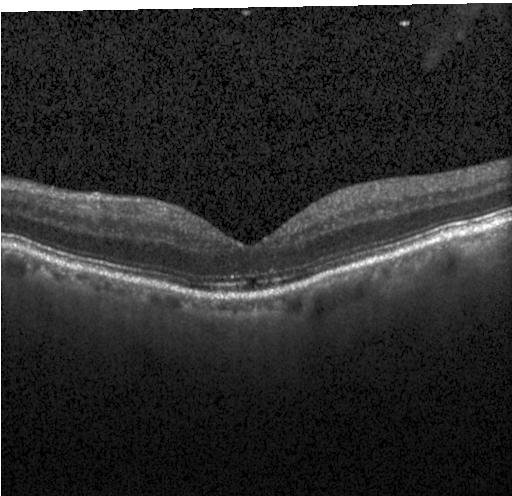 OCT line scan · Heidelberg Spectralis OCT system · macular scan · spectral-domain optical coherence tomography
Diagnosis: no choroidal neovascularization, diabetic macular edema, or drusen.